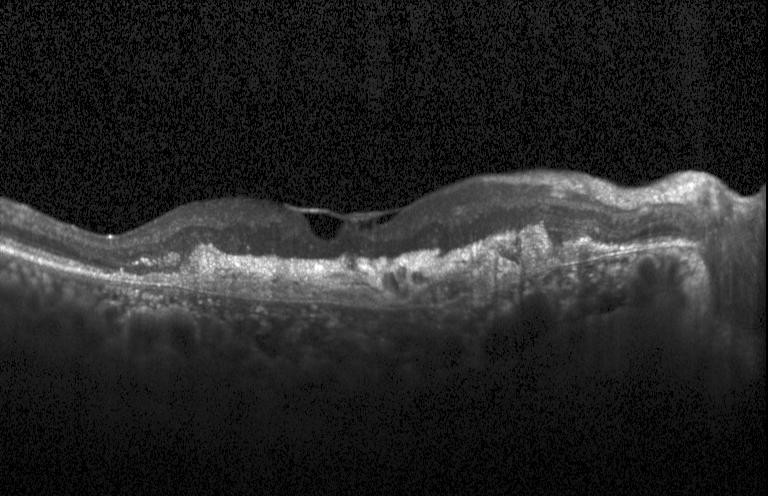

Heidelberg Spectralis OCT system; retinal OCT cross-section; spectral-domain optical coherence tomography.
A choroidal neovascular membrane.